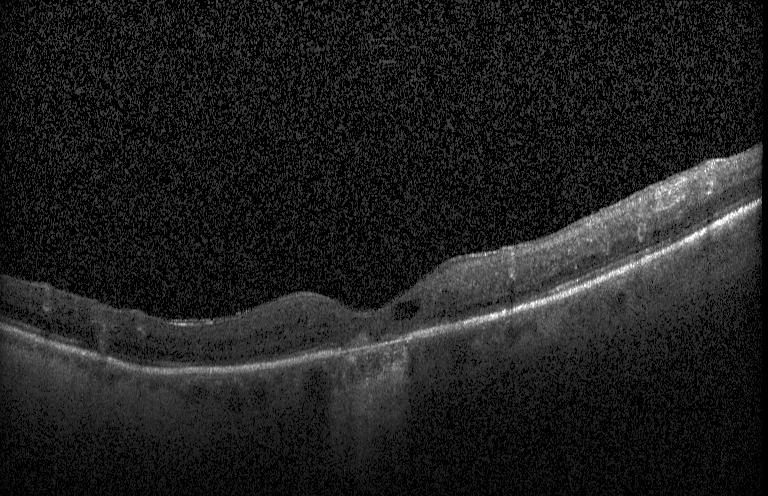 Finding: choroidal neovascularization (CNV).